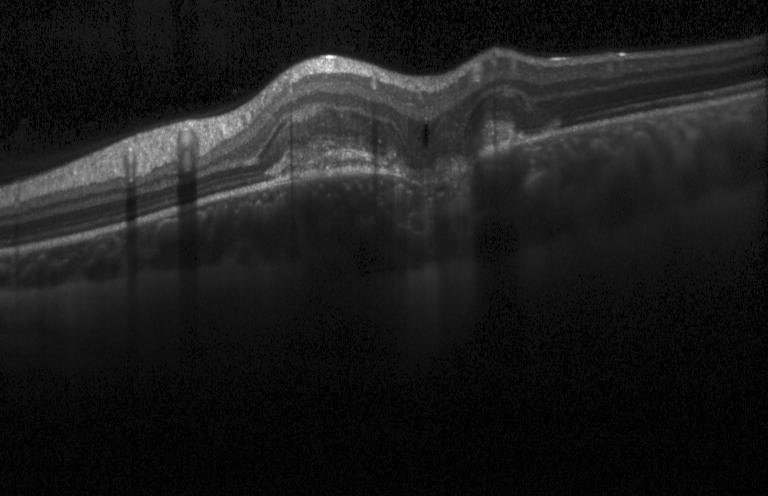 Optical coherence tomography B-scan, spectral-domain OCT, acquired on a Heidelberg Spectralis. This B-scan demonstrates a choroidal neovascular membrane.